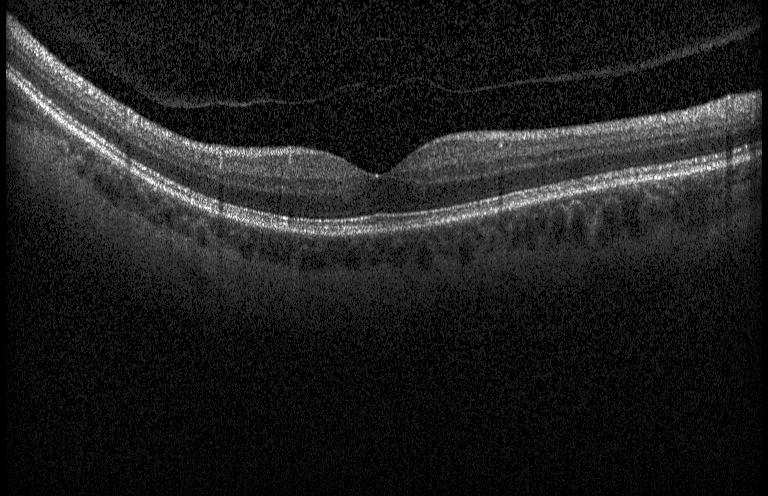
Retinal OCT cross-section, acquired on a Heidelberg Spectralis.
Macular OCT: neither choroidal neovascularization, diabetic macular edema, nor drusen.